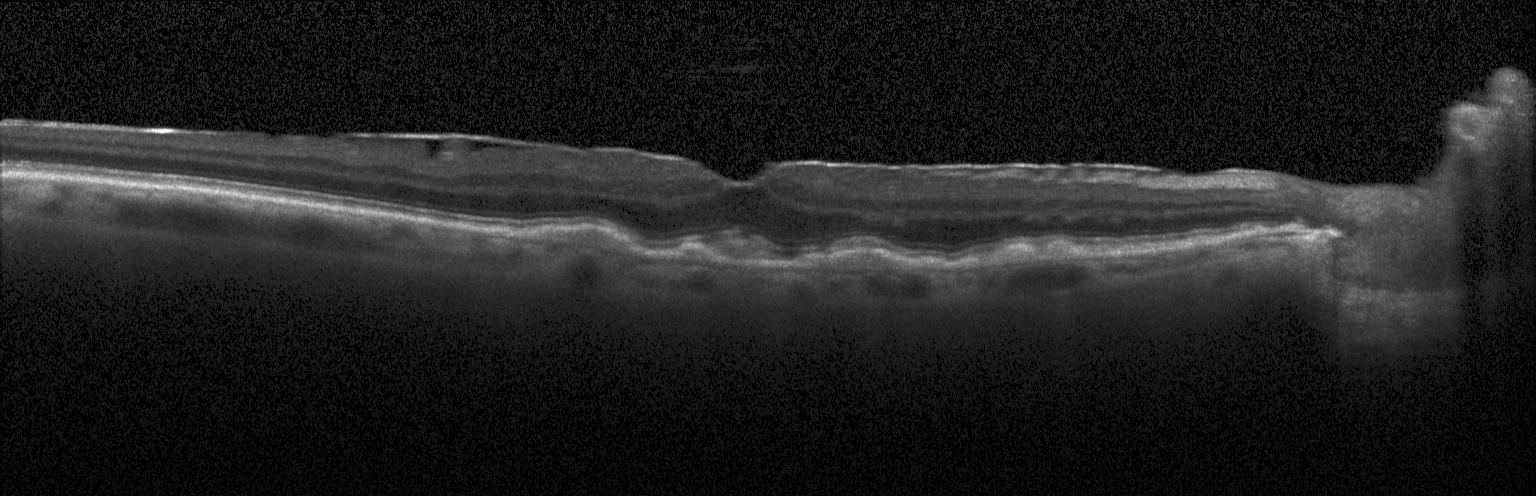

OCT B-scan; instrument: Heidelberg Spectralis. OCT finding: sub-RPE drusenoid deposits.